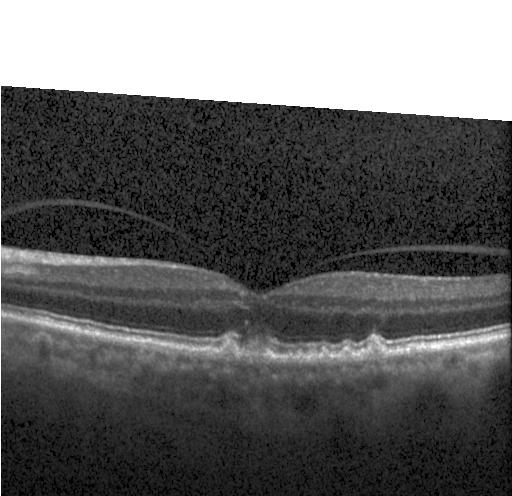

OCT B-scan, macular scan, SD-OCT — Finding: drusen.